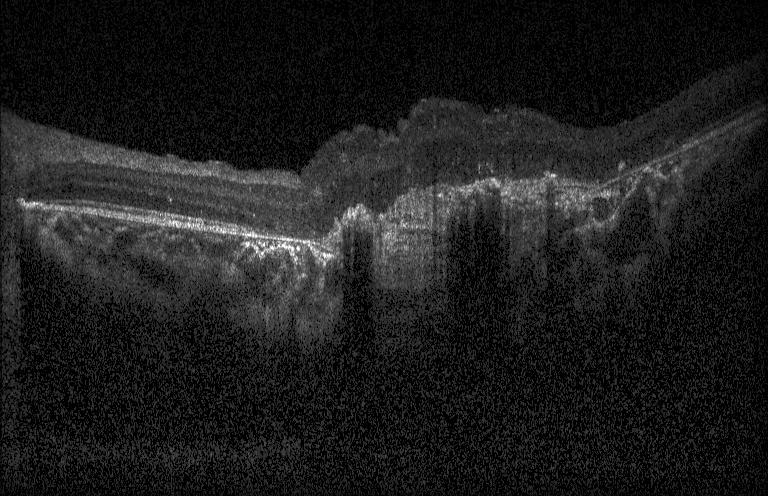
SD-OCT · Heidelberg Spectralis OCT system · centered on the fovea · optical coherence tomography scan. OCT finding: choroidal neovascularization (CNV).